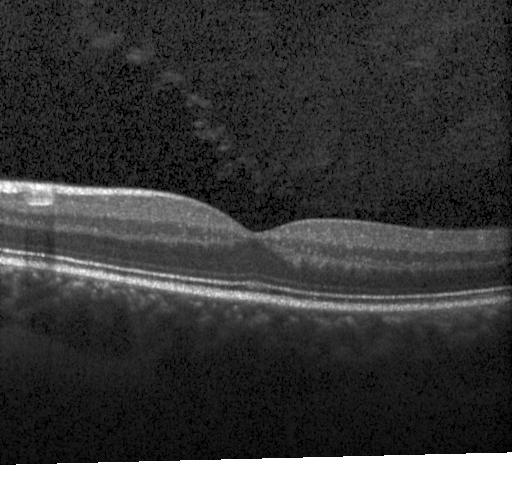 Optical coherence tomography scan · SD-OCT. OCT finding: no evidence of choroidal neovascularization, diabetic macular edema, or drusen.